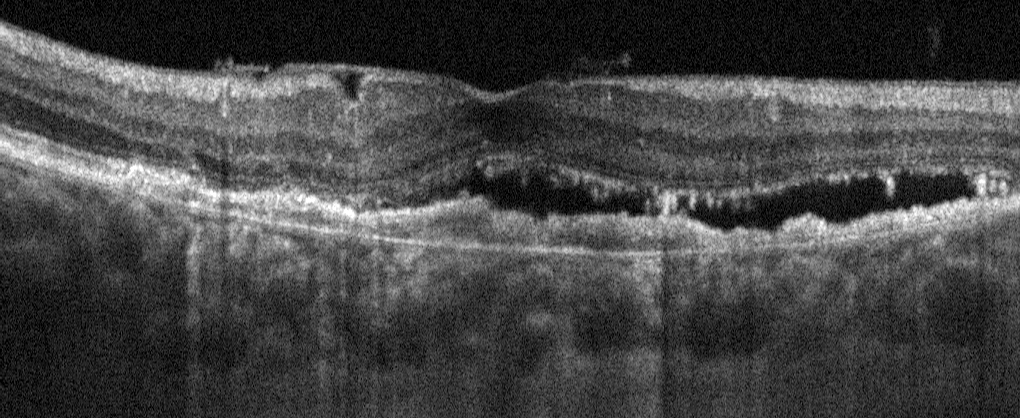

Diagnosis: AMD.